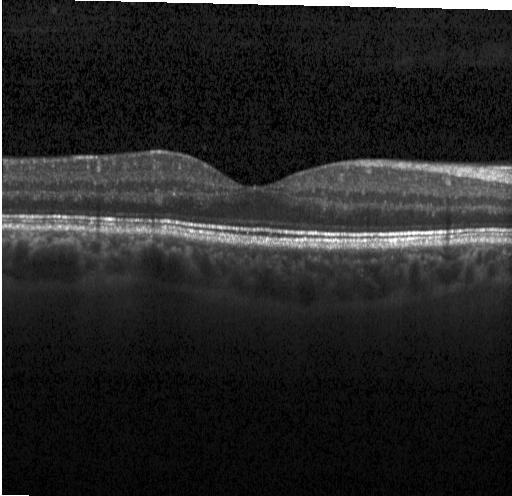 Finding: no evidence of choroidal neovascularization, diabetic macular edema, or drusen.